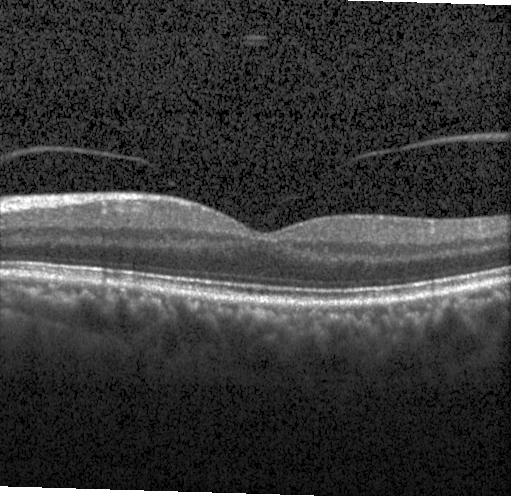 Heidelberg Spectralis · OCT B-scan · SD-OCT · fovea-centered.
This B-scan demonstrates no evidence of CNV, DME, or drusen.